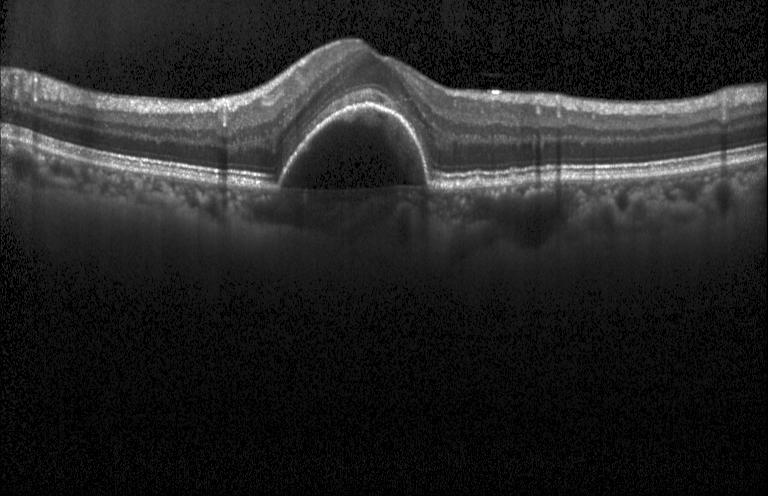 OCT B-scan showing a choroidal neovascular membrane.